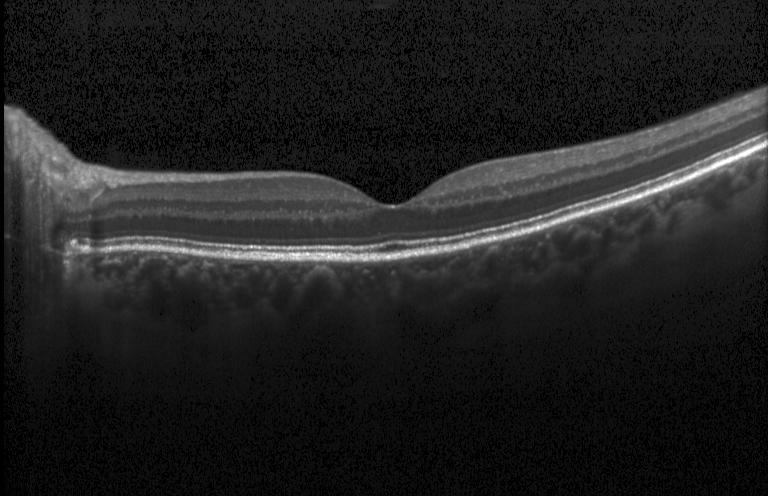 Dx: no CNV, DME, or drusen.